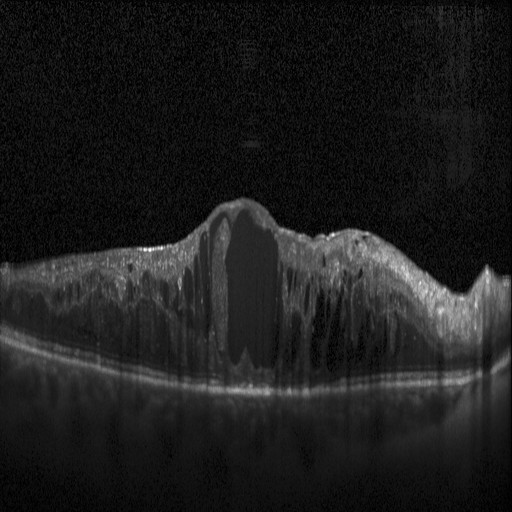 OCT line scan
Diagnosis: DME.